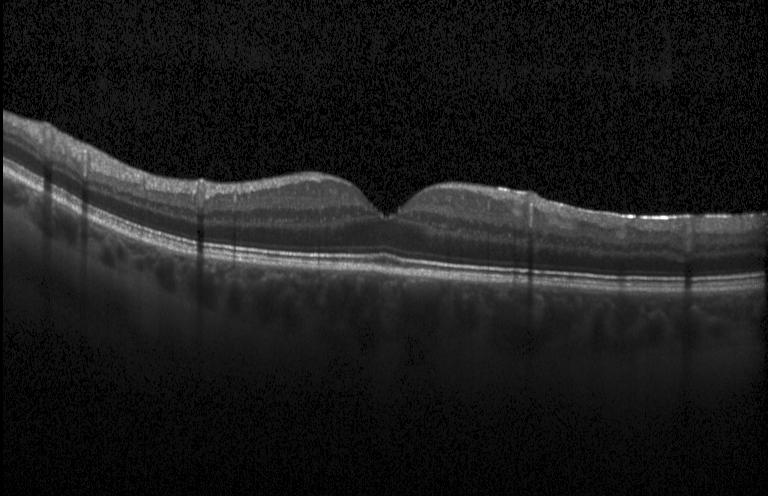

Through the macula · optical coherence tomography B-scan · SD-OCT
This B-scan demonstrates no CNV, DME, or drusen.